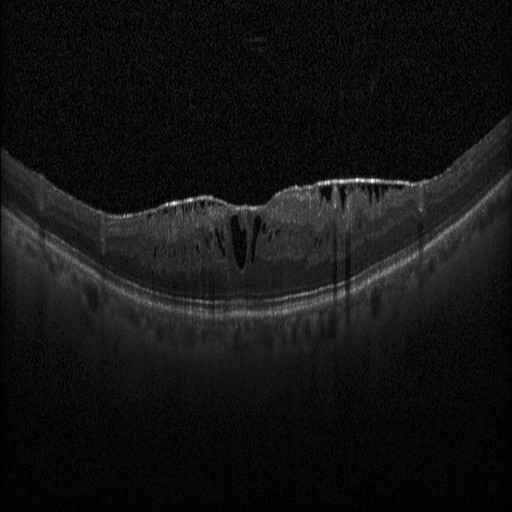
Retinal OCT B-scan, acquired on a Heidelberg Spectralis, spectral-domain optical coherence tomography
The scan shows diabetic macular edema.